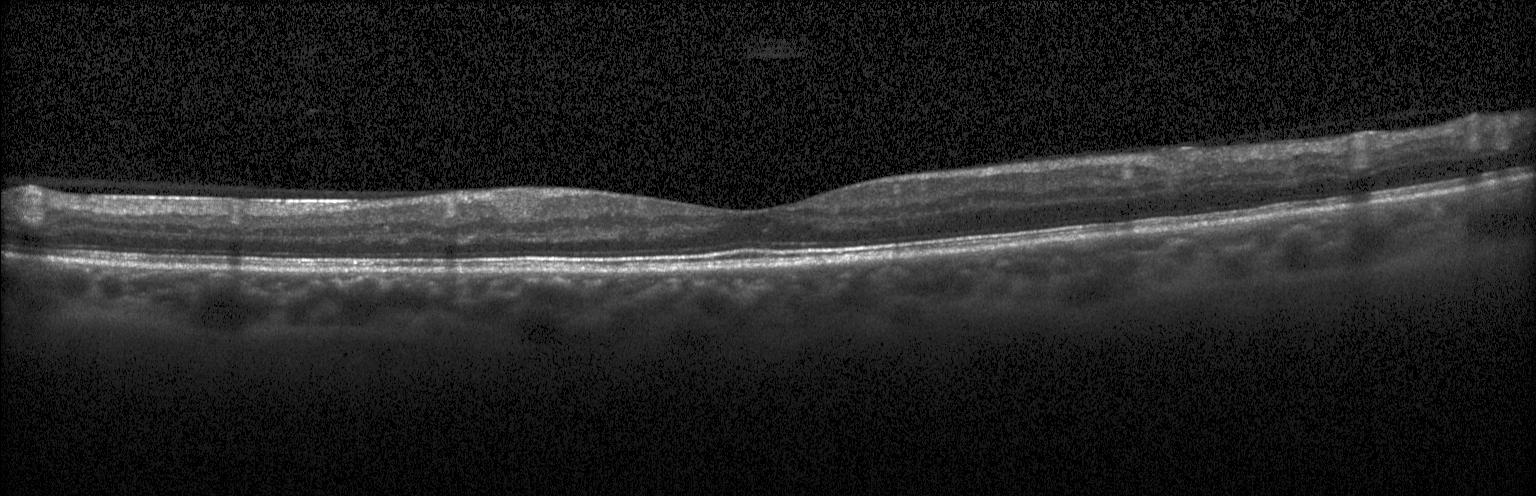
SD-OCT; Heidelberg Spectralis; optical coherence tomography B-scan. OCT finding: neither CNV, DME, nor drusen.